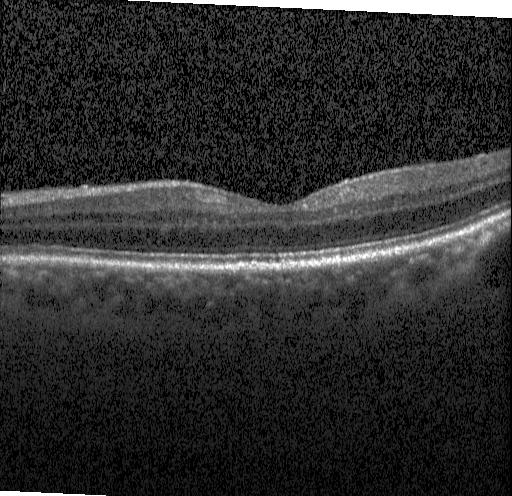 OCT finding: neither choroidal neovascularization, diabetic macular edema, nor drusen.